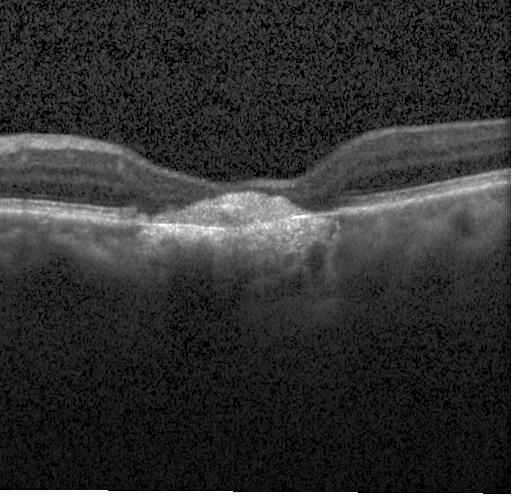
Spectral-domain optical coherence tomography, retinal OCT cross-section, Heidelberg Spectralis OCT system. Finding: CNV.